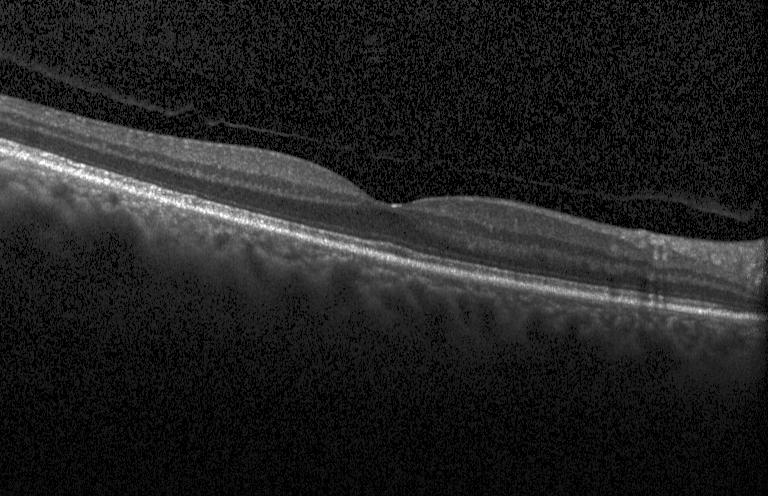
OCT B-scan showing no evidence of CNV, DME, or drusen.